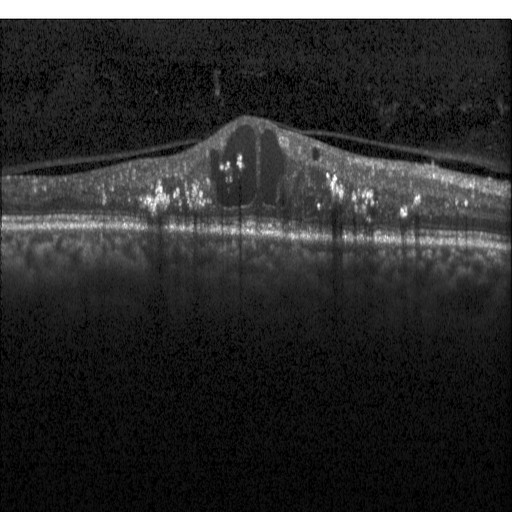
OCT B-scan, Heidelberg Spectralis, spectral-domain optical coherence tomography — This B-scan demonstrates DME.